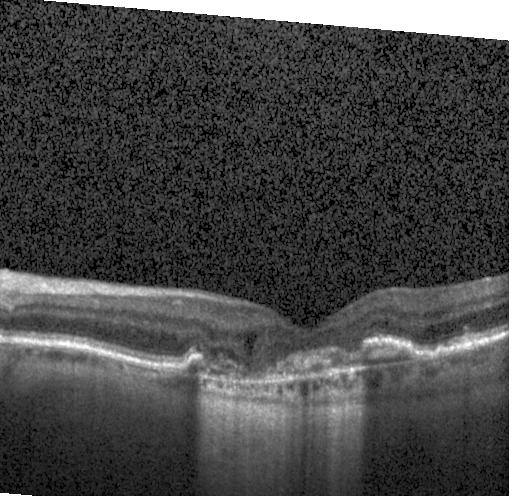 OCT B-scan; macular scan.
The scan shows choroidal neovascularization.